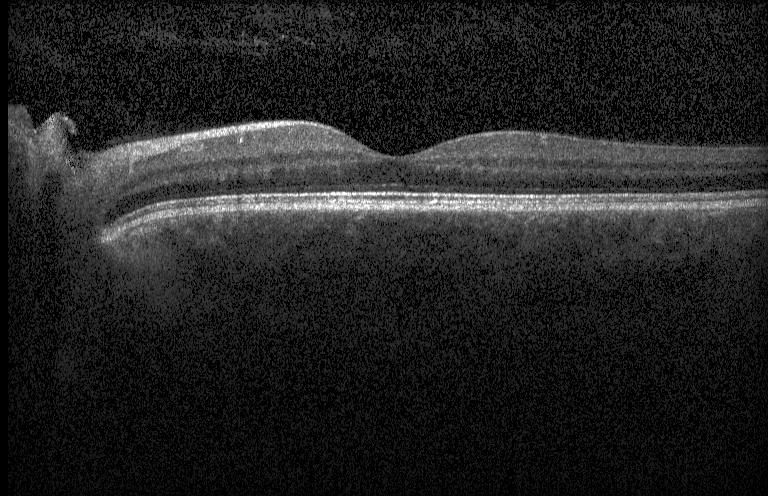 OCT finding: no choroidal neovascularization, no diabetic macular edema, and no drusen.